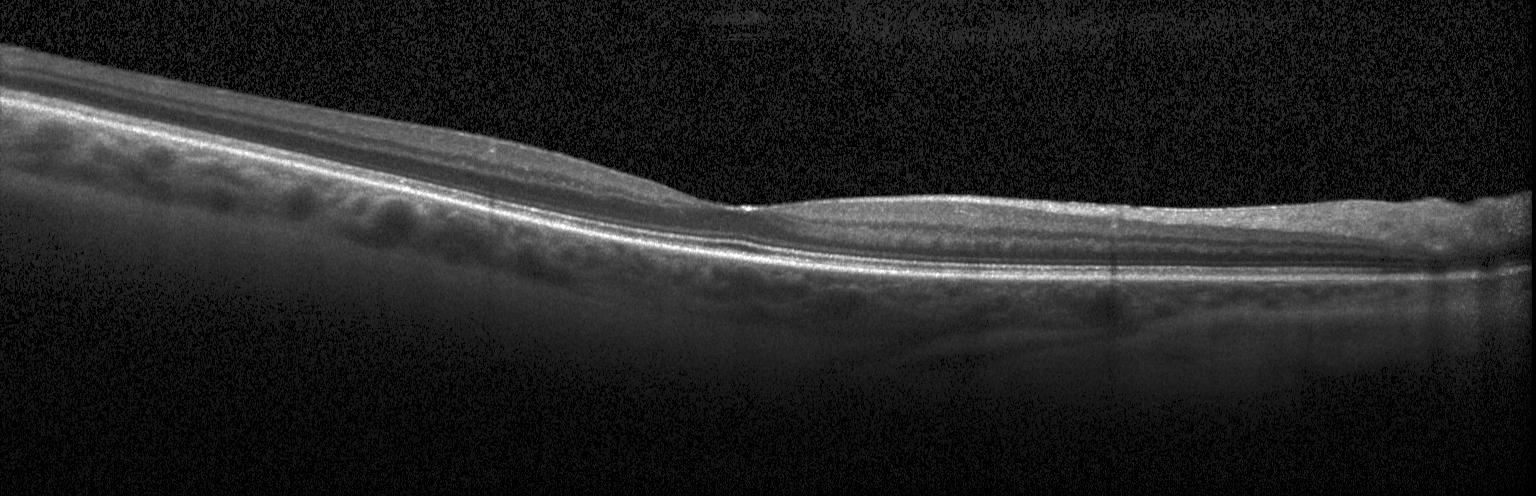
Spectral-domain OCT. Retinal OCT cross-section. Through the macula — OCT finding: no evidence of choroidal neovascularization, diabetic macular edema, or drusen.